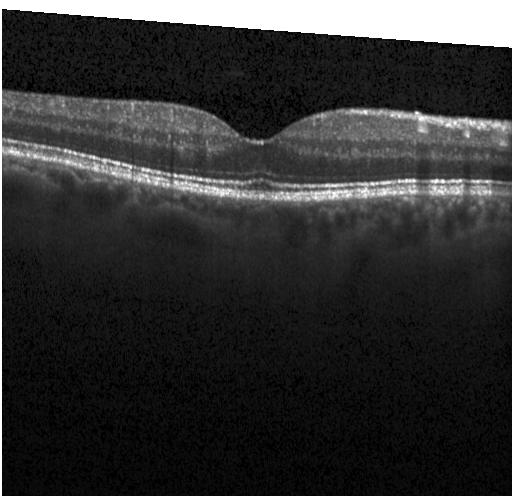 OCT line scan · spectral-domain optical coherence tomography · Heidelberg Spectralis OCT system · macular scan — Diagnosis: no choroidal neovascularization, no diabetic macular edema, and no drusen.